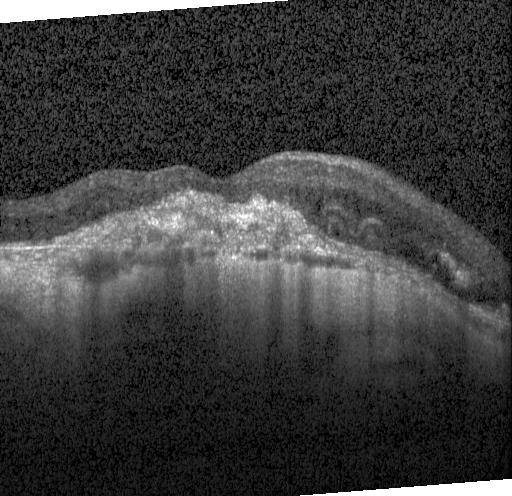 Optical coherence tomography scan. Spectral-domain OCT. Instrument: Heidelberg Spectralis.
Macular OCT: choroidal neovascularization (CNV).